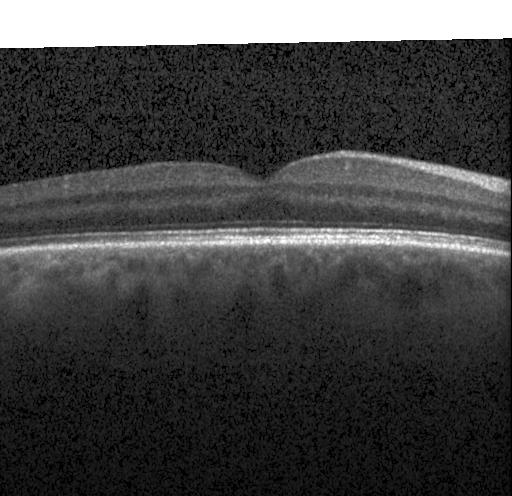

Diagnosis: no CNV, no DME, and no drusen.